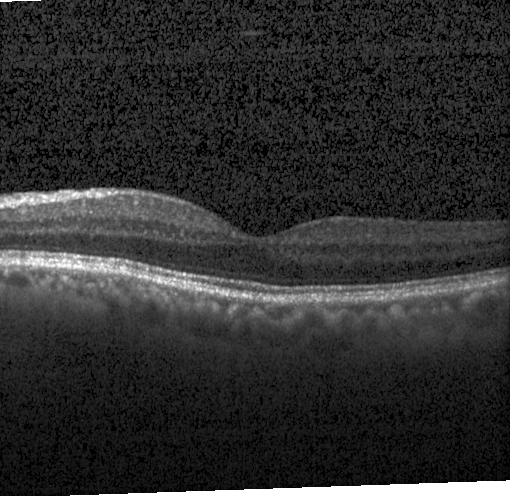 Acquired on a Heidelberg Spectralis. Retinal OCT B-scan — Diagnosis: no choroidal neovascularization, diabetic macular edema, or drusen.